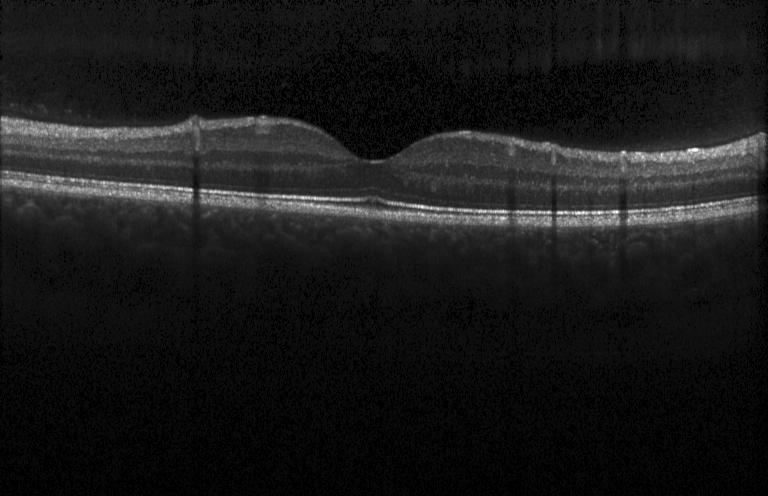 Retinal OCT B-scan — Finding: no choroidal neovascularization, no diabetic macular edema, and no drusen.